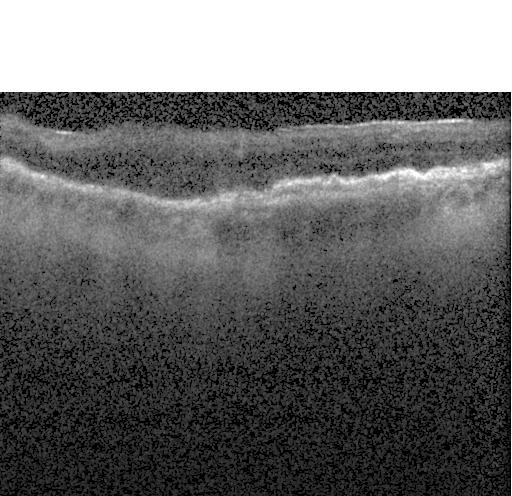
Retinal OCT cross-section · Heidelberg Spectralis OCT system · SD-OCT
Assessment: a choroidal neovascular membrane.